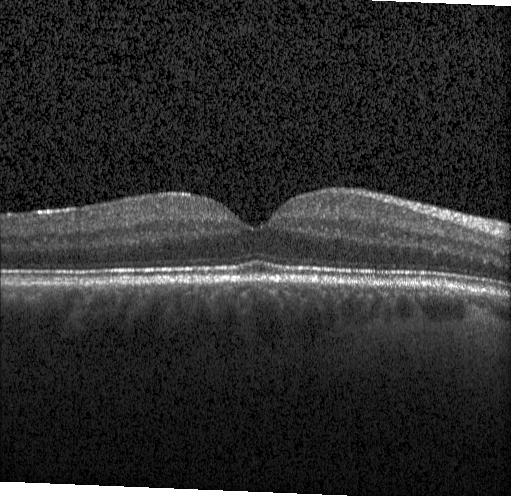

Optical coherence tomography B-scan; acquired on a Heidelberg Spectralis; spectral-domain optical coherence tomography
Impression: no choroidal neovascularization, no diabetic macular edema, and no drusen.